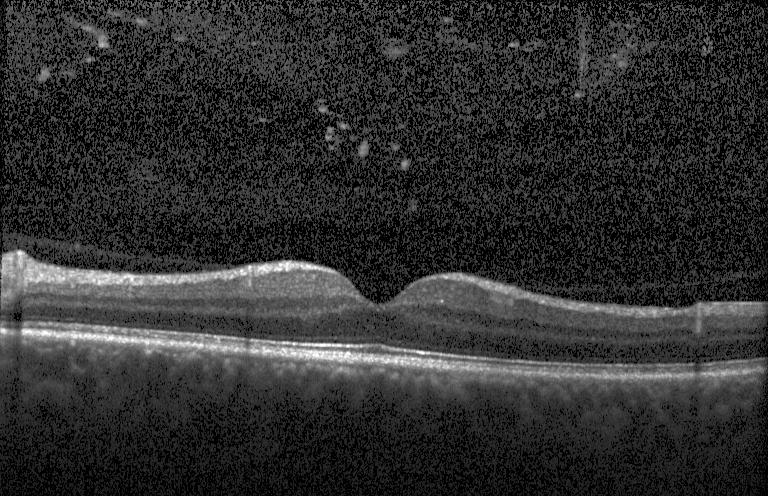 Impression: no CNV, DME, or drusen.